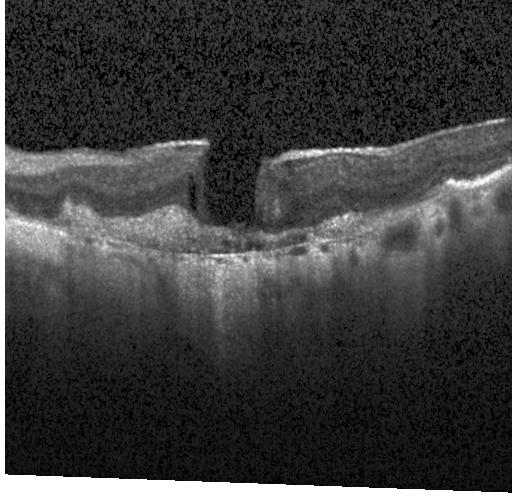

Acquired on a Heidelberg Spectralis. Retinal OCT B-scan. Spectral-domain OCT
This B-scan demonstrates choroidal neovascularization (CNV).